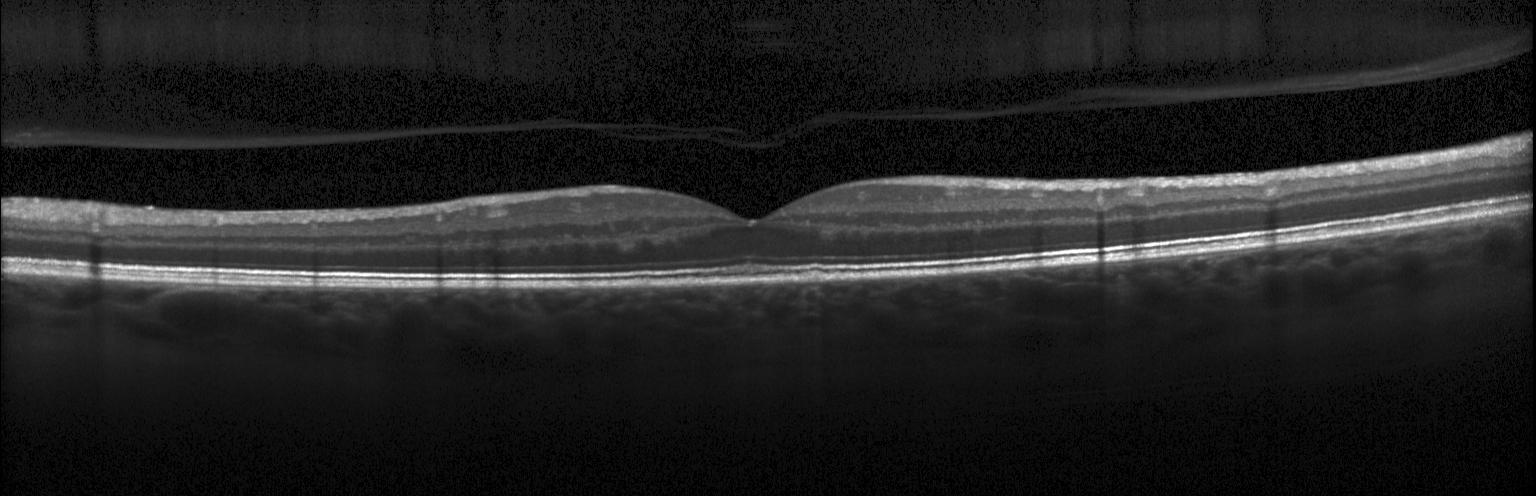

Horizontal scan through the fovea, OCT line scan, spectral-domain optical coherence tomography, Heidelberg Spectralis OCT system
Diagnosis: no evidence of choroidal neovascularization, diabetic macular edema, or drusen.